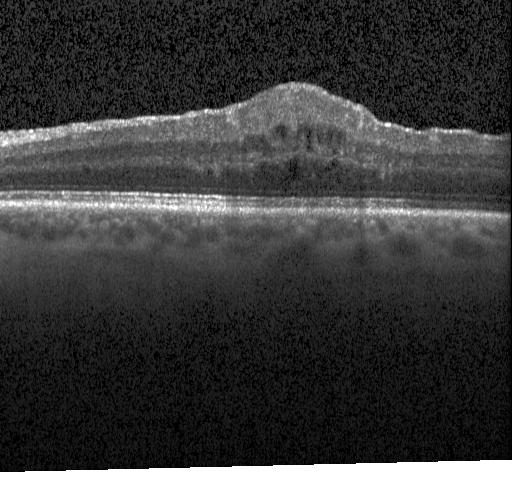

Retinal OCT B-scan.
The scan shows diabetic macular edema.